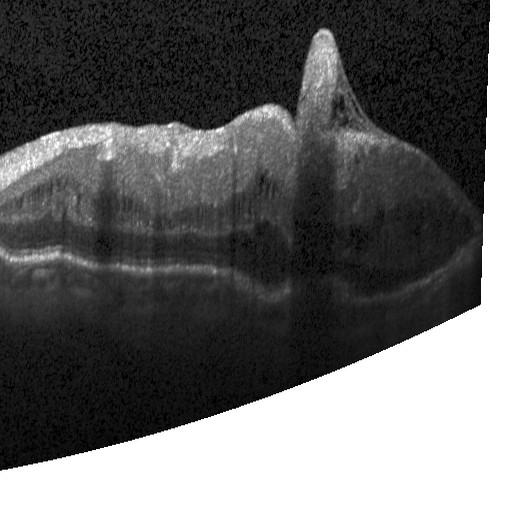

Retinal OCT cross-section.
Diabetic macular edema (DME).